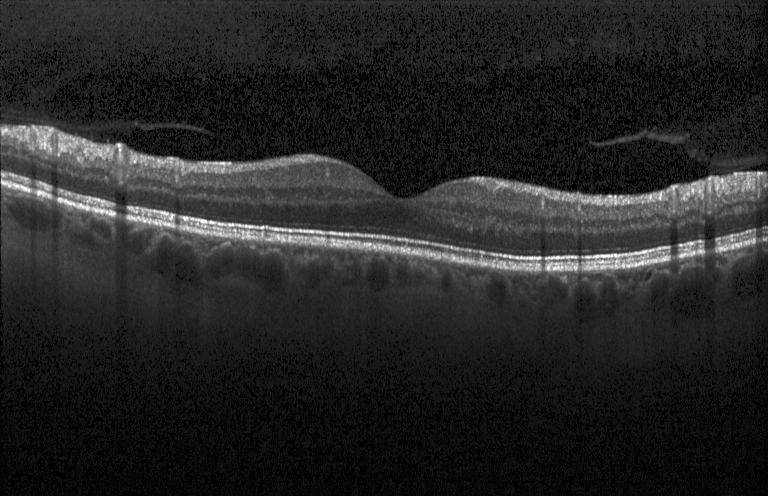 Heidelberg Spectralis OCT system. Spectral-domain optical coherence tomography. Optical coherence tomography B-scan. Diagnosis: neither choroidal neovascularization, diabetic macular edema, nor drusen.